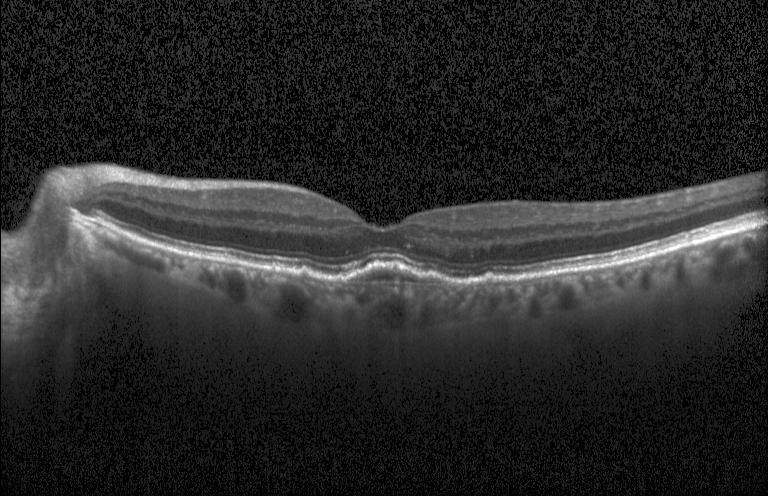

Spectral-domain OCT, optical coherence tomography B-scan, Heidelberg Spectralis OCT system
Impression: a choroidal neovascular membrane.